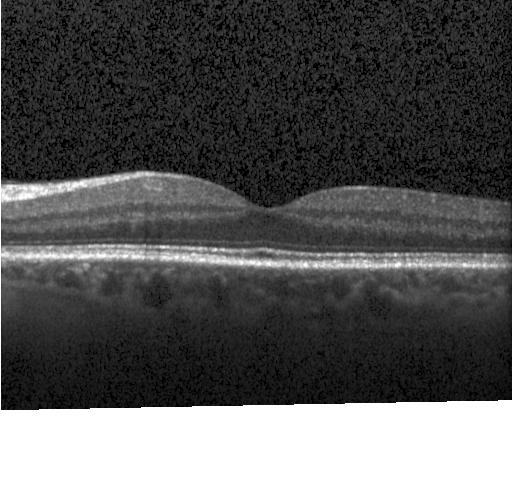
Retinal OCT B-scan.
Assessment: no evidence of CNV, DME, or drusen.